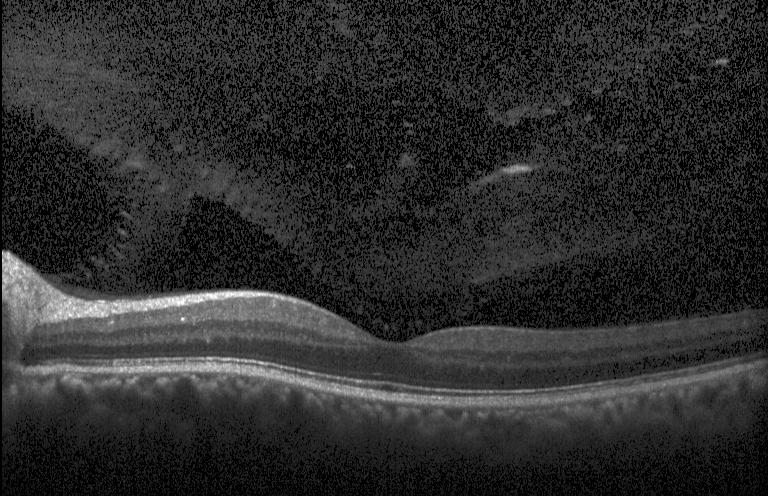 Instrument: Heidelberg Spectralis · optical coherence tomography scan · macular scan · SD-OCT. Finding: neither CNV, DME, nor drusen.